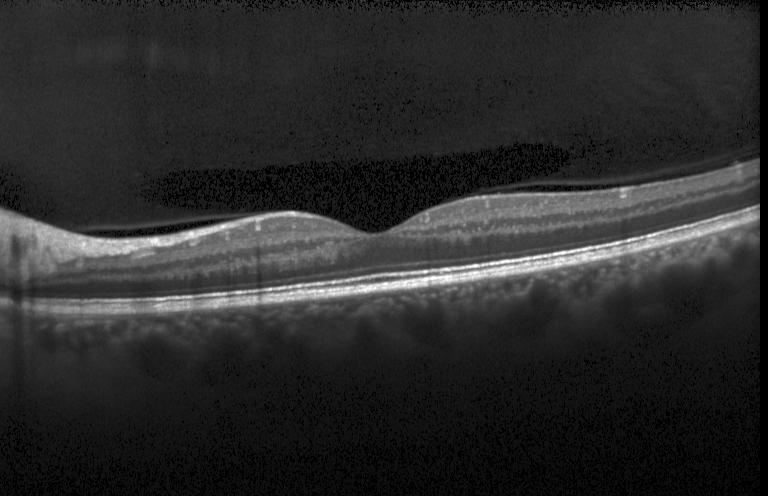

Impression: no evidence of CNV, DME, or drusen.